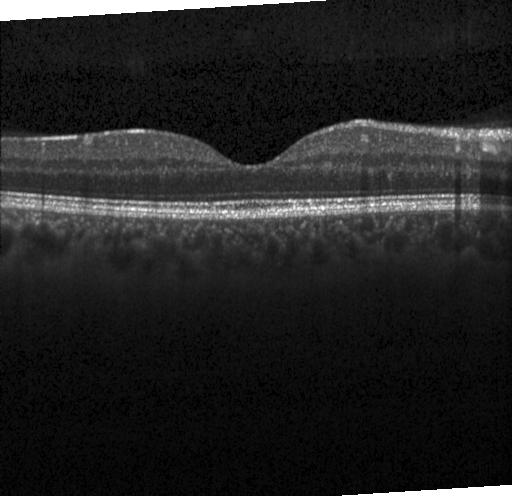
Spectral-domain optical coherence tomography; retinal OCT cross-section; horizontal scan through the fovea — Finding: neither CNV, DME, nor drusen.